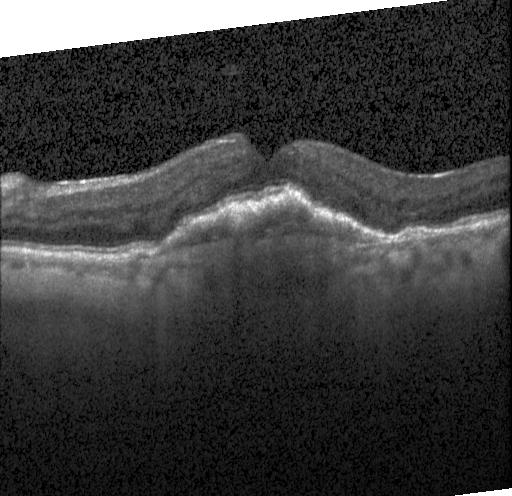
Retinal OCT B-scan · SD-OCT · instrument: Heidelberg Spectralis · macular scan.
OCT finding: a choroidal neovascular membrane.